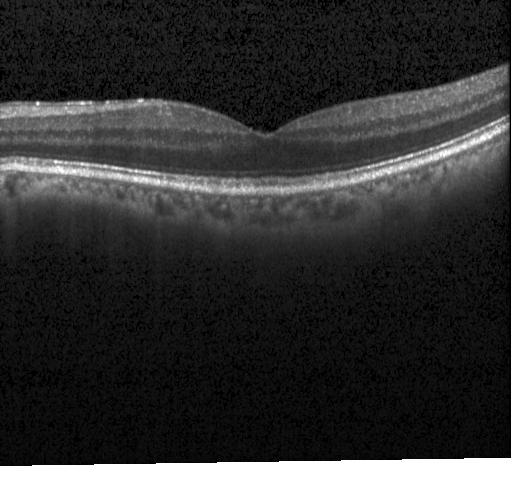

Optical coherence tomography B-scan, spectral-domain OCT, instrument: Heidelberg Spectralis. Diagnosis: no evidence of choroidal neovascularization, diabetic macular edema, or drusen.